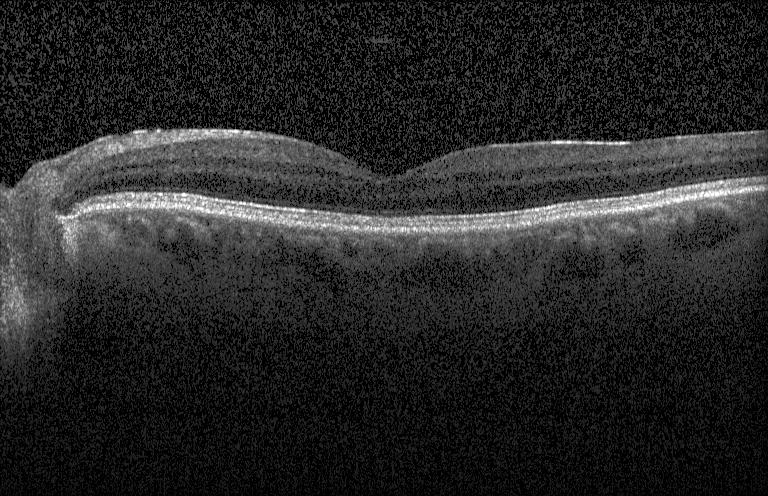
Heidelberg Spectralis · OCT line scan
No choroidal neovascularization, no diabetic macular edema, and no drusen.